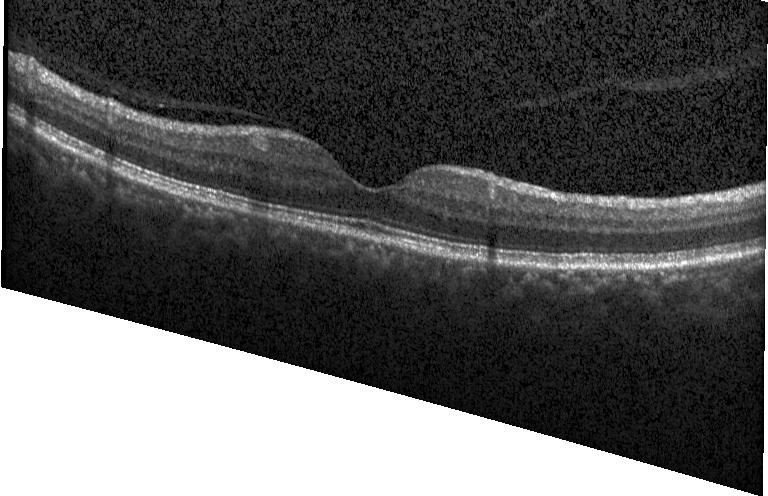 OCT line scan. Centered on the fovea. Acquired on a Heidelberg Spectralis. Macular OCT: no evidence of CNV, DME, or drusen.